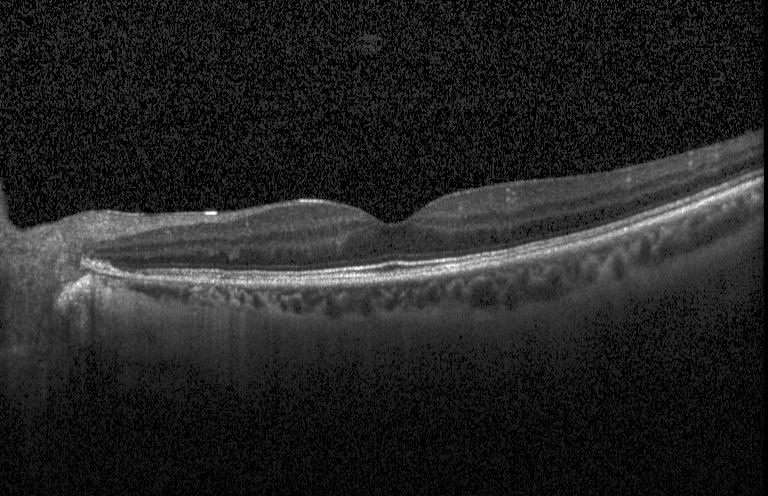 Optical coherence tomography scan — Assessment: no evidence of choroidal neovascularization, diabetic macular edema, or drusen.